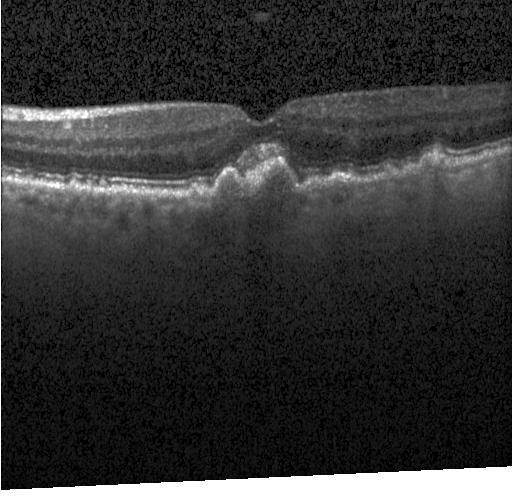

Heidelberg Spectralis. Macular scan. Spectral-domain OCT. Retinal OCT B-scan. Impression: a choroidal neovascular membrane.